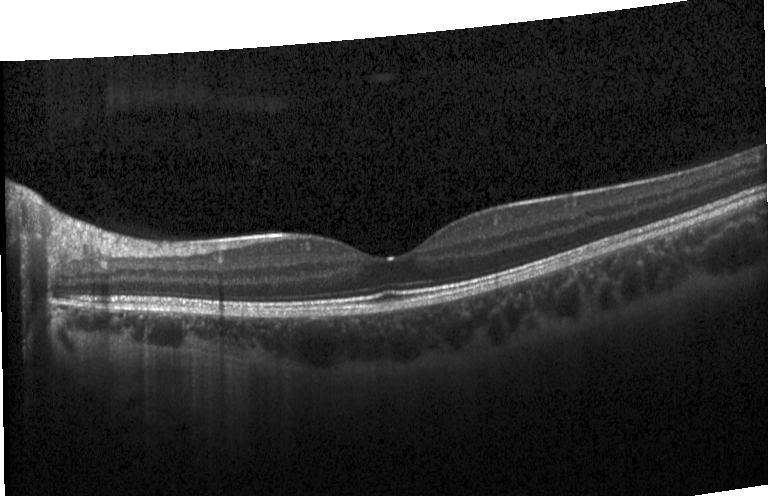
OCT line scan — Finding: neither choroidal neovascularization, diabetic macular edema, nor drusen.